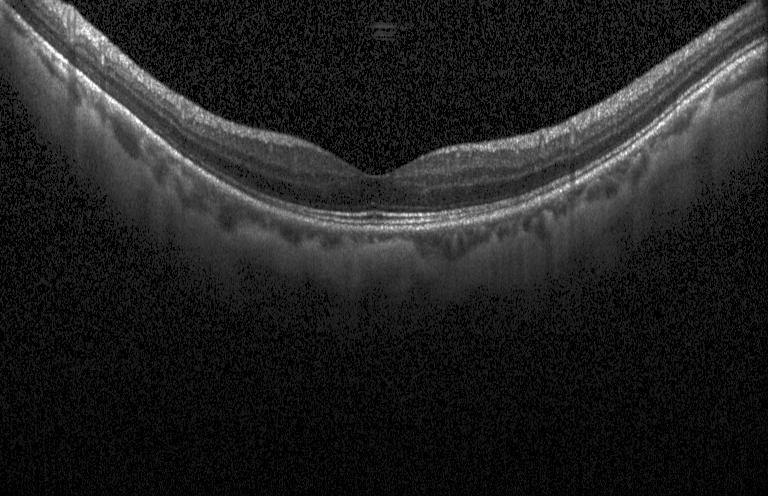

Macular OCT: no evidence of choroidal neovascularization, diabetic macular edema, or drusen.